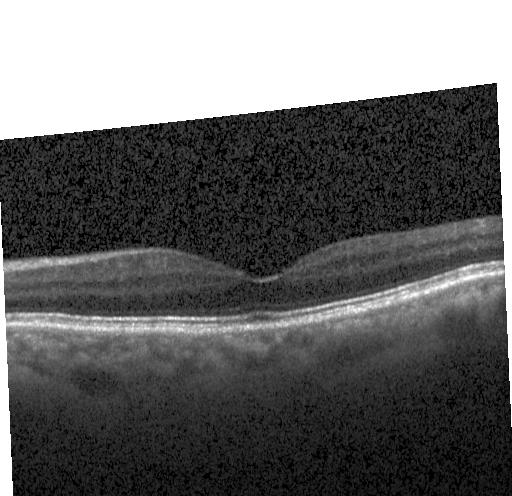 Optical coherence tomography B-scan — Finding: no evidence of choroidal neovascularization, diabetic macular edema, or drusen.